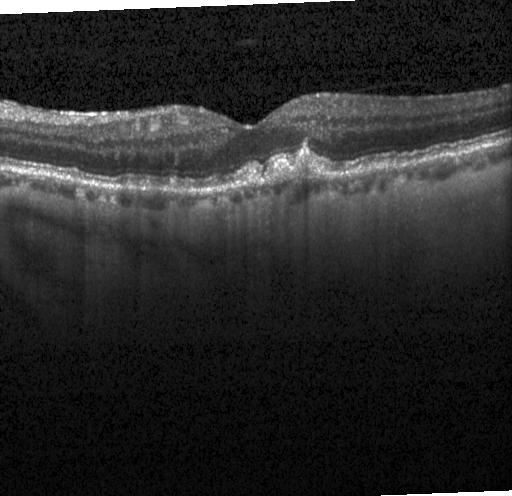

OCT line scan; SD-OCT; horizontal scan through the fovea; acquired on a Heidelberg Spectralis — This B-scan demonstrates sub-RPE drusenoid deposits.